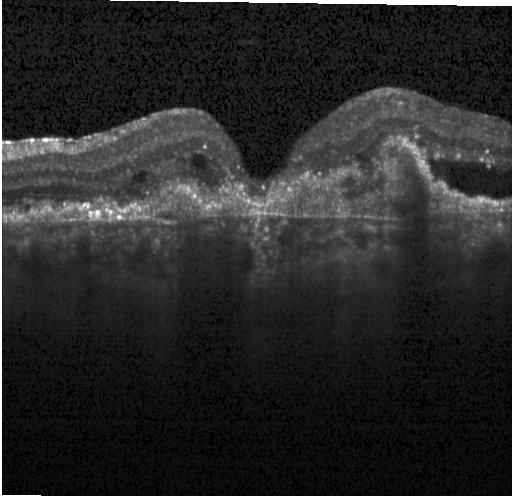
Through the macula. Heidelberg Spectralis. Optical coherence tomography B-scan. Spectral-domain optical coherence tomography — Finding: CNV.